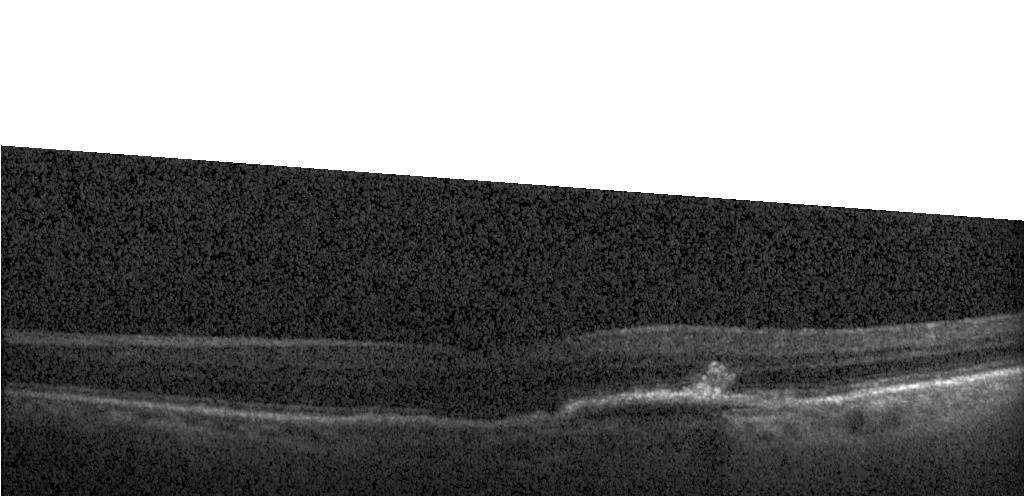 Impression: choroidal neovascularization (CNV).